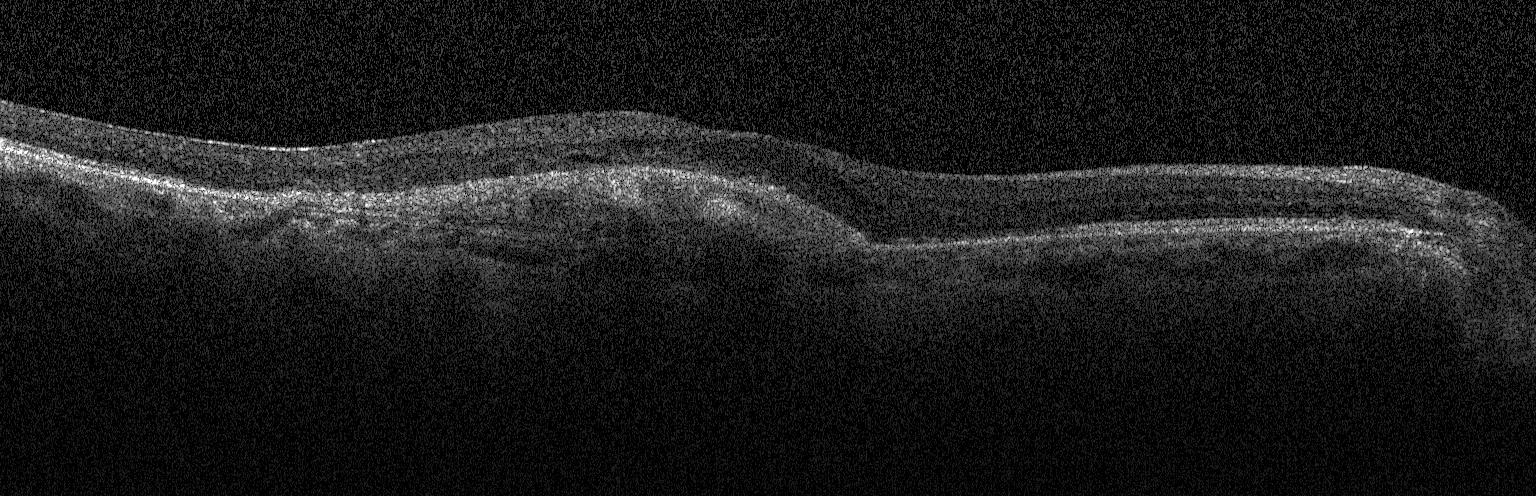

Spectral-domain optical coherence tomography. Acquired on a Heidelberg Spectralis. Retinal OCT cross-section. Fovea-centered
Diagnosis: CNV.